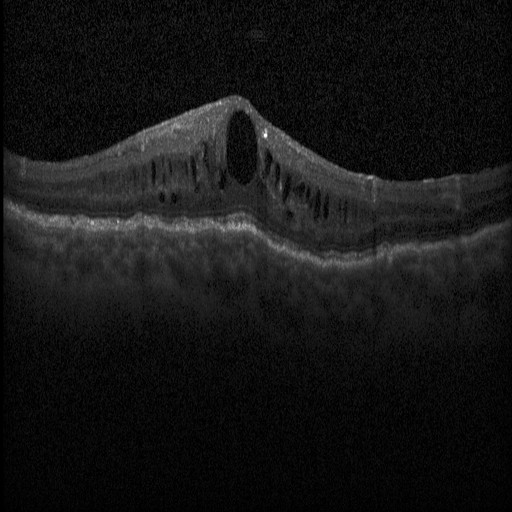 OCT line scan. Spectral-domain OCT. Through the macula. Heidelberg Spectralis OCT system. Diabetic macular edema (DME).